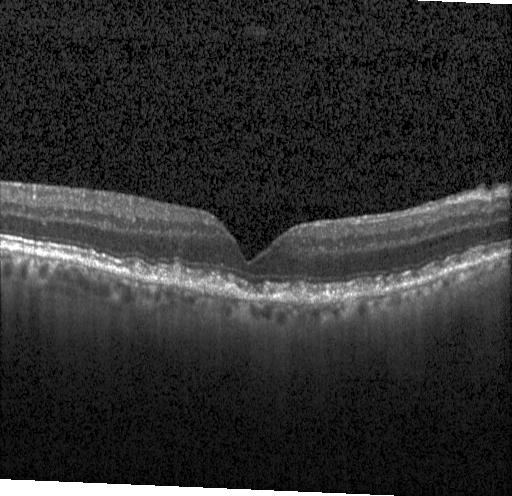 SD-OCT. Optical coherence tomography scan. Through the macula. Acquired on a Heidelberg Spectralis
Finding: multiple drusen.